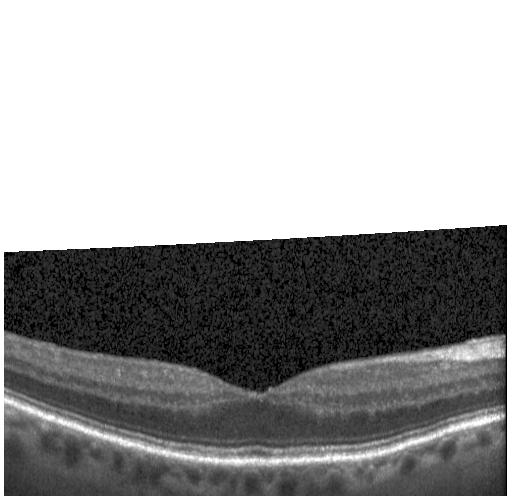 Dx: no choroidal neovascularization, no diabetic macular edema, and no drusen.